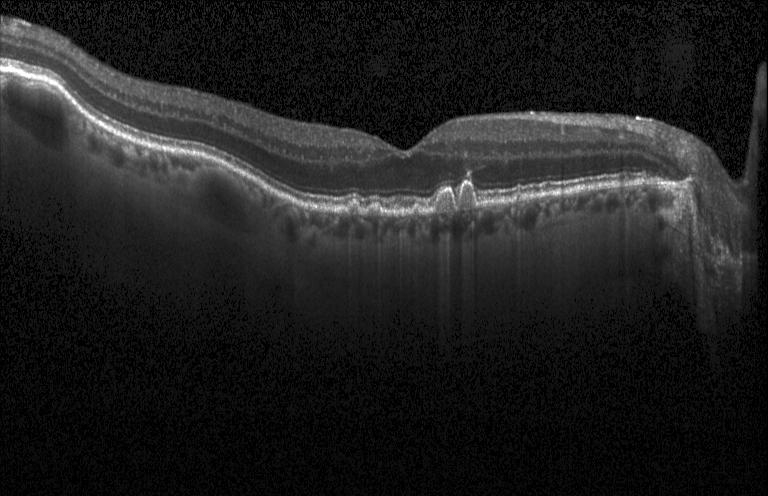
Drusen.